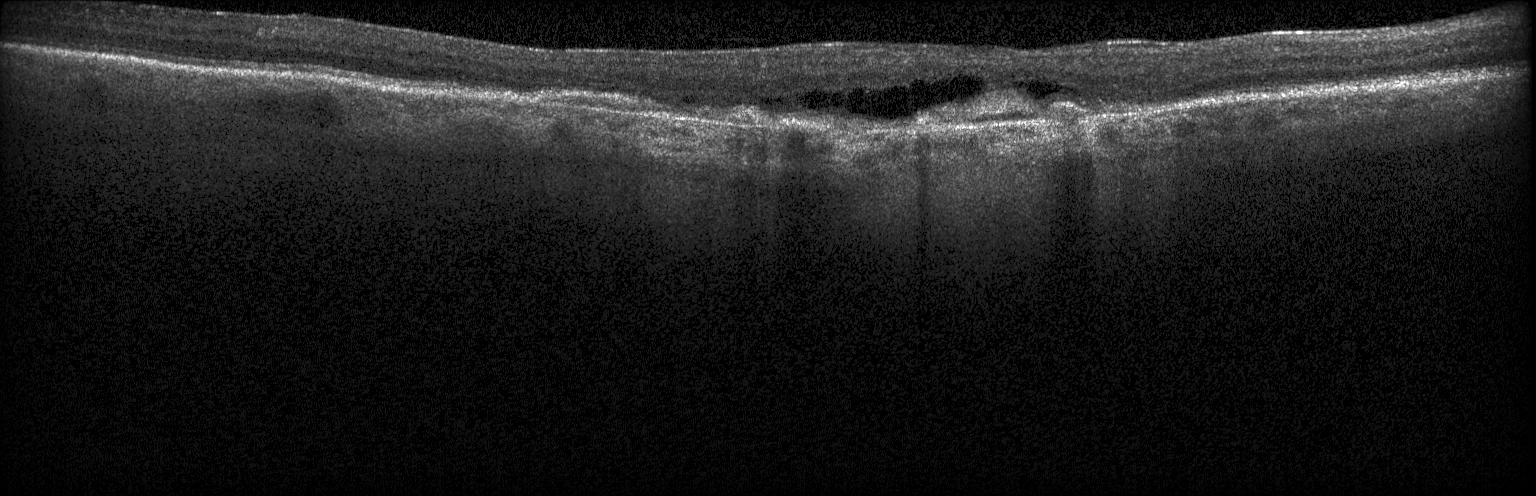
OCT line scan · macular scan. A choroidal neovascular membrane.